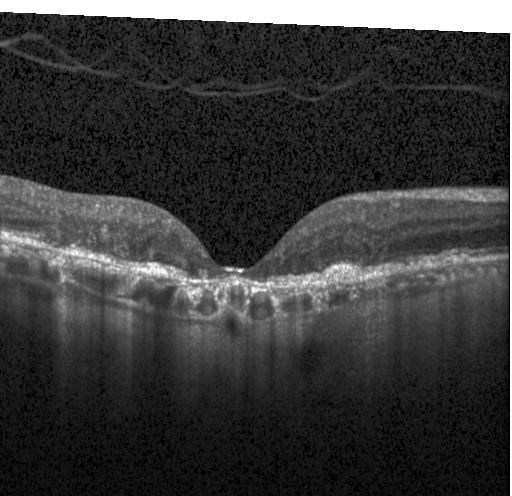

Spectral-domain OCT B-scan: choroidal neovascularization.